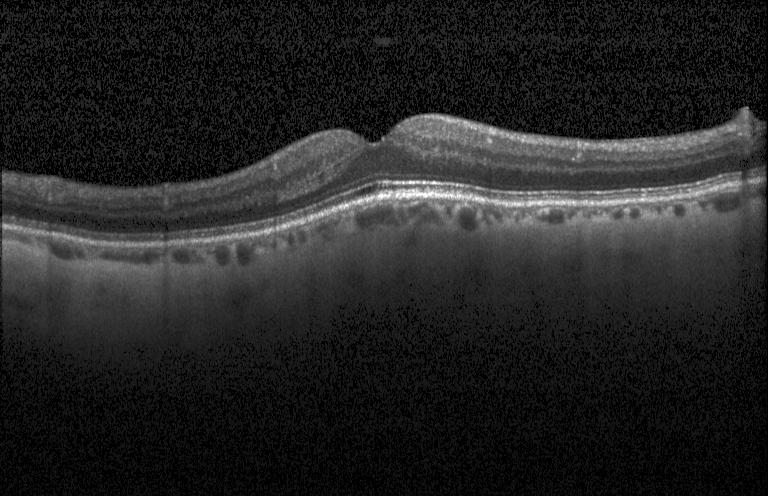
OCT scan showing neither choroidal neovascularization, diabetic macular edema, nor drusen.